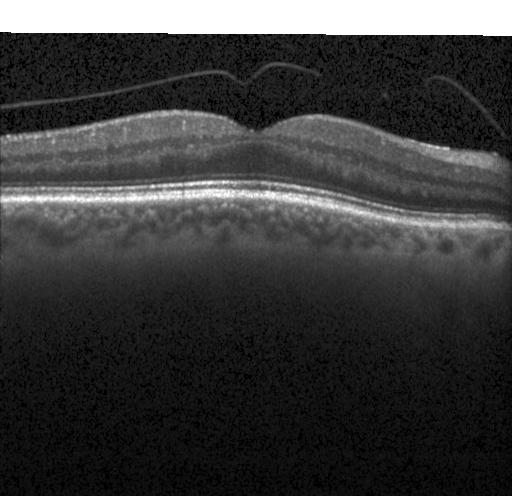

OCT B-scan — Diagnosis: no evidence of CNV, DME, or drusen.